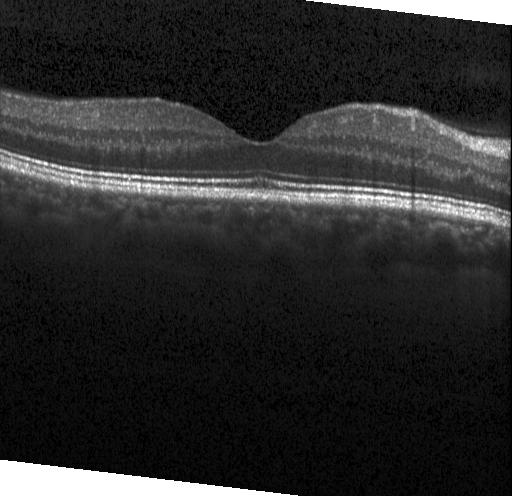 Diagnosis: no choroidal neovascularization, diabetic macular edema, or drusen.